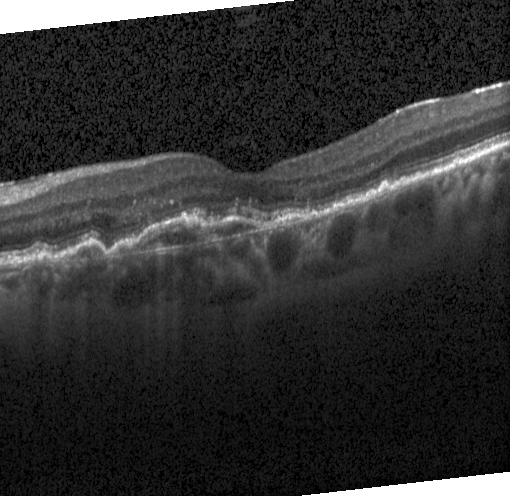

Instrument: Heidelberg Spectralis · spectral-domain optical coherence tomography · OCT B-scan
Diagnosis: a choroidal neovascular membrane.